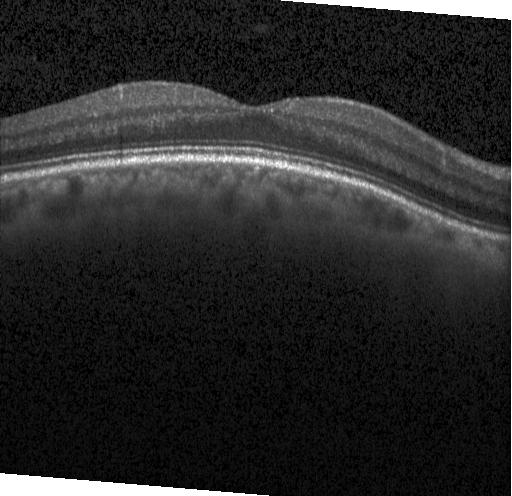
OCT scan showing no evidence of choroidal neovascularization, diabetic macular edema, or drusen.